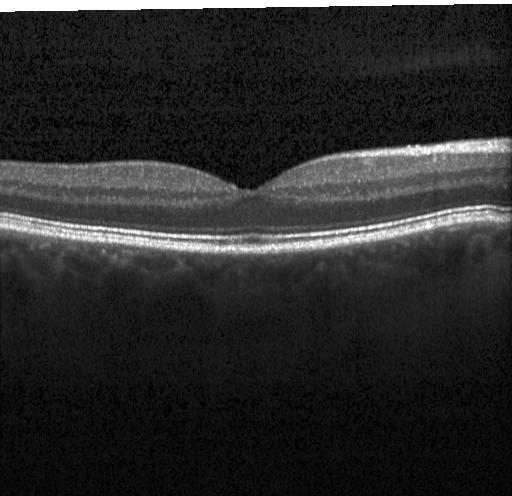

OCT line scan — Diagnosis: no evidence of choroidal neovascularization, diabetic macular edema, or drusen.